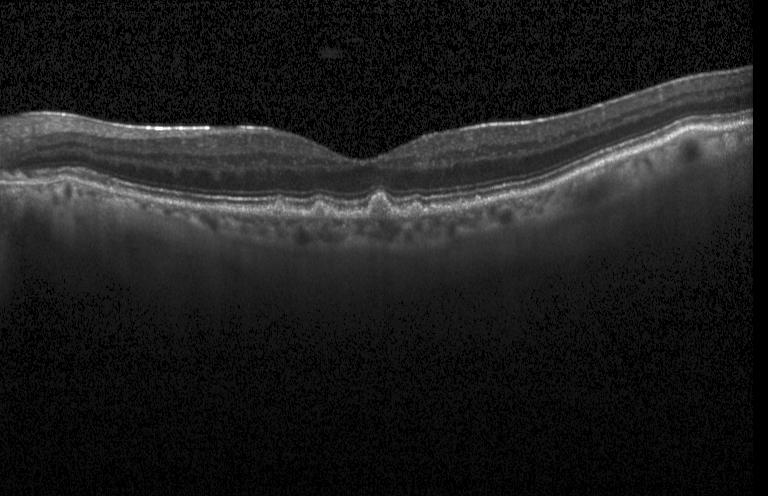

OCT line scan
Assessment: multiple drusen.